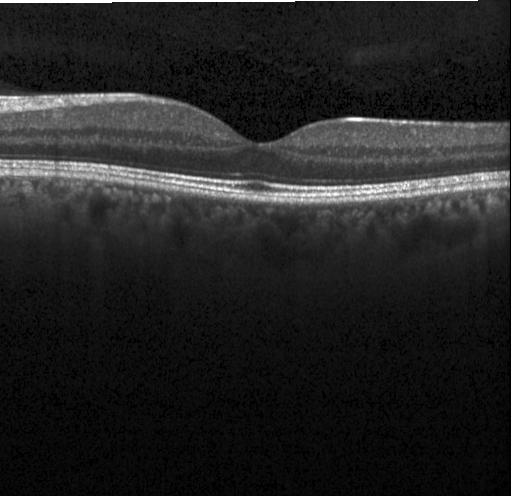

OCT finding: no evidence of CNV, DME, or drusen.